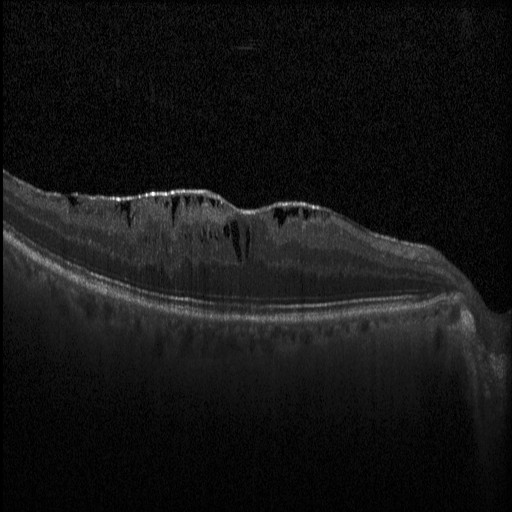 Macular OCT: DME.